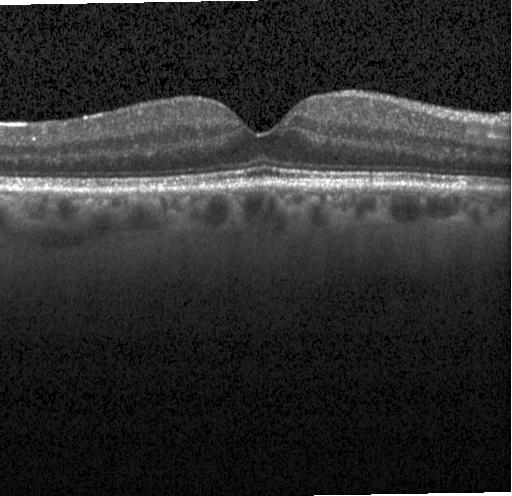

OCT B-scan, spectral-domain OCT, horizontal scan through the fovea, Heidelberg Spectralis OCT system. Impression: no CNV, DME, or drusen.